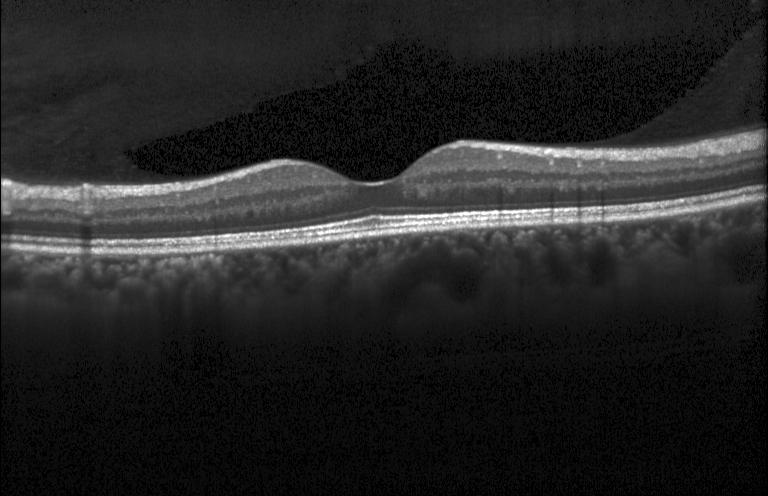

Centered on the fovea; OCT B-scan; spectral-domain optical coherence tomography
Impression: no choroidal neovascularization, diabetic macular edema, or drusen.